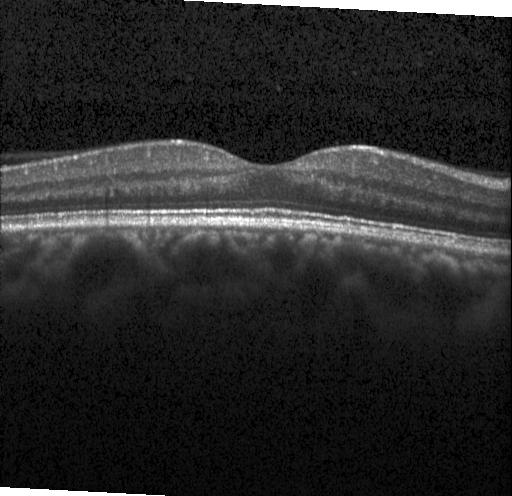 Macular OCT: no evidence of CNV, DME, or drusen.